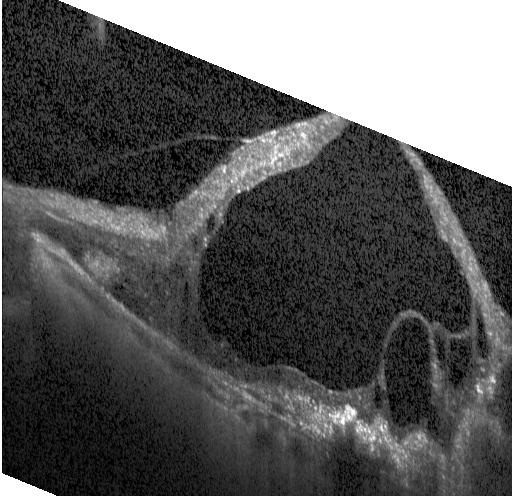

Acquired on a Heidelberg Spectralis; optical coherence tomography B-scan.
Finding: choroidal neovascularization (CNV).